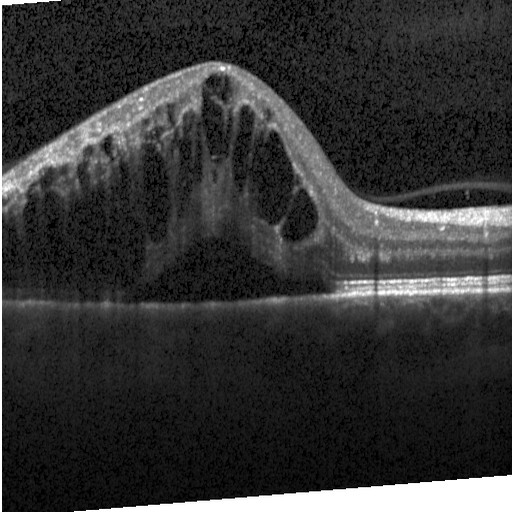 Spectral-domain OCT B-scan: DME.